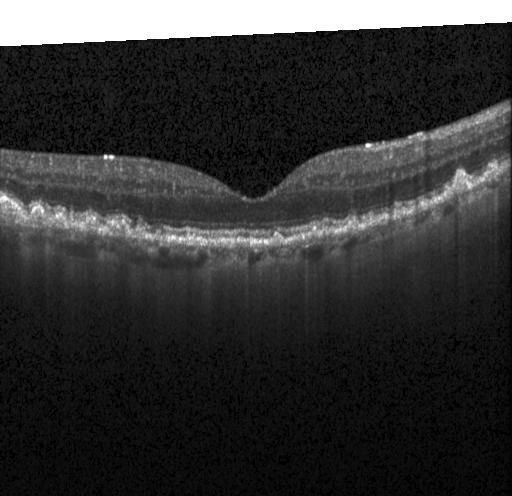 OCT scan showing drusen.